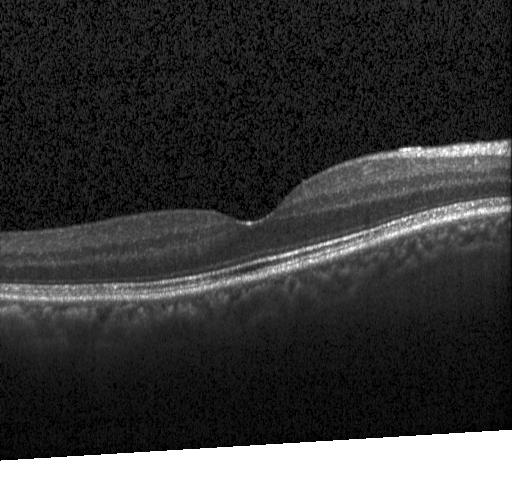 This B-scan demonstrates no choroidal neovascularization, diabetic macular edema, or drusen.